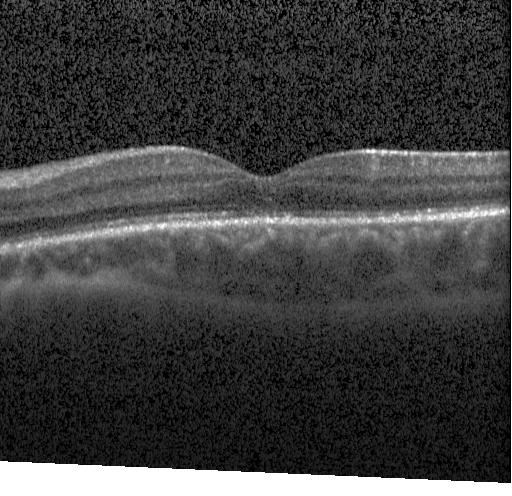
Optical coherence tomography B-scan. Spectral-domain OCT. Assessment: no choroidal neovascularization, diabetic macular edema, or drusen.